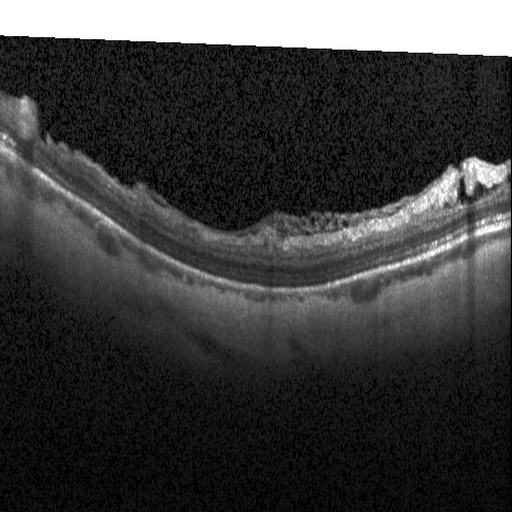
Impression: diabetic macular edema (DME).